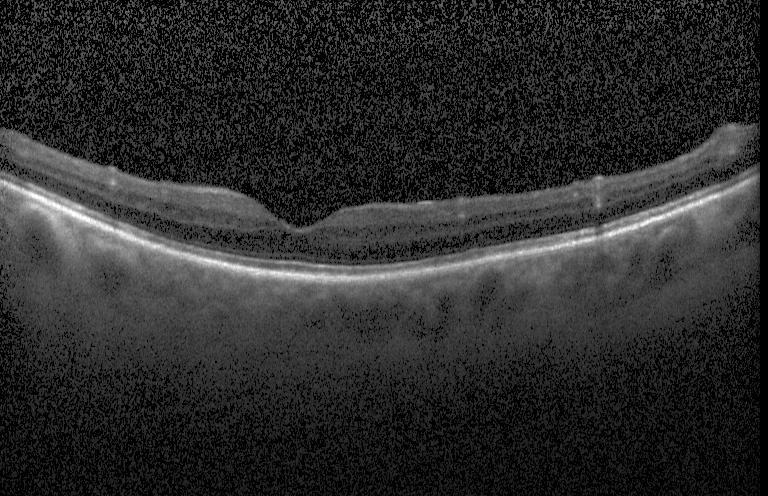

Optical coherence tomography B-scan — Impression: no CNV, DME, or drusen.